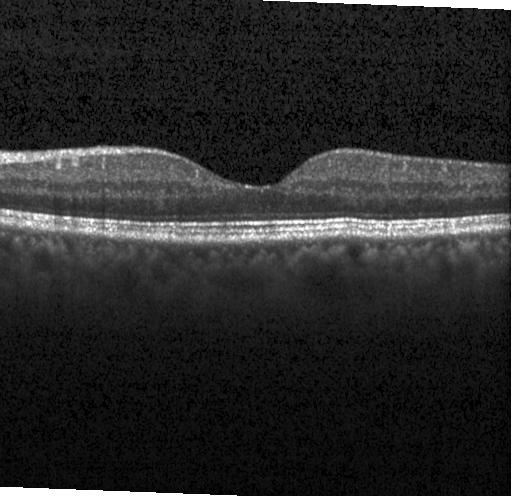 OCT line scan · fovea-centered · instrument: Heidelberg Spectralis
Macular OCT: neither CNV, DME, nor drusen.